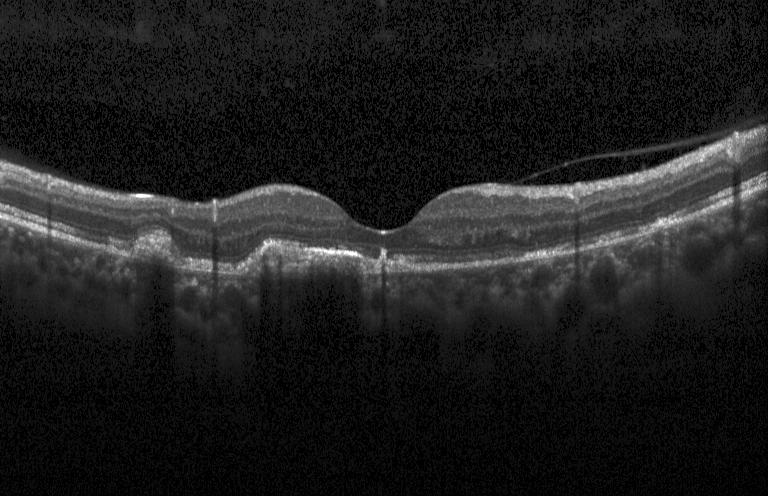 Heidelberg Spectralis, through the macula, OCT line scan — Diagnosis: choroidal neovascularization (CNV).